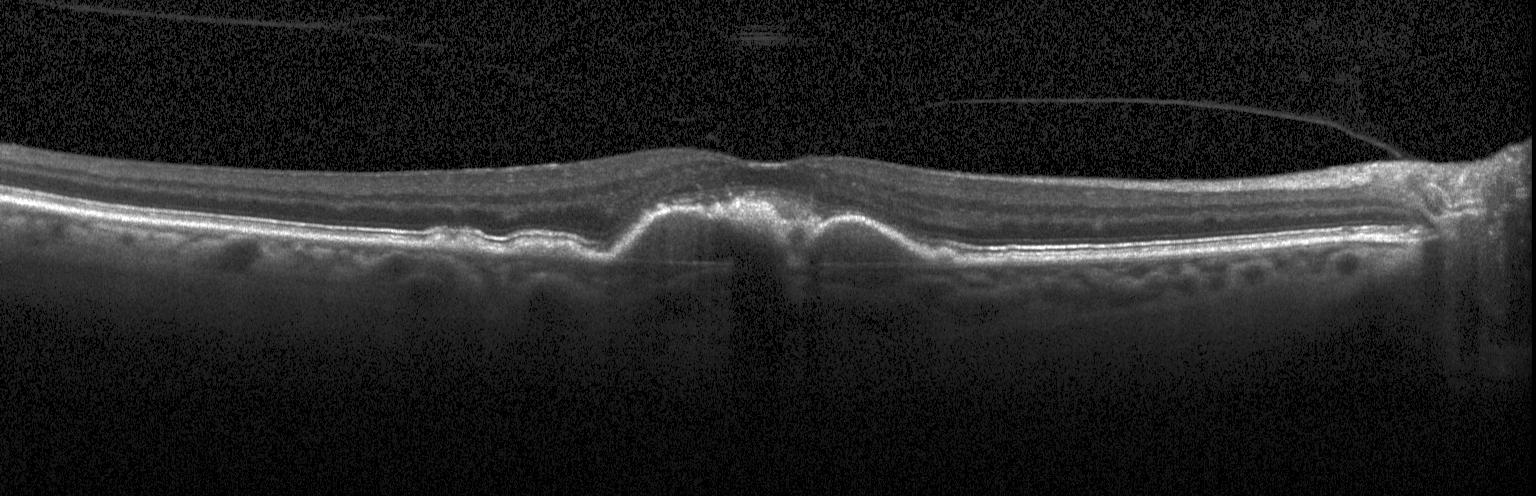 Spectral-domain optical coherence tomography · fovea-centered · OCT B-scan.
This B-scan demonstrates a choroidal neovascular membrane.